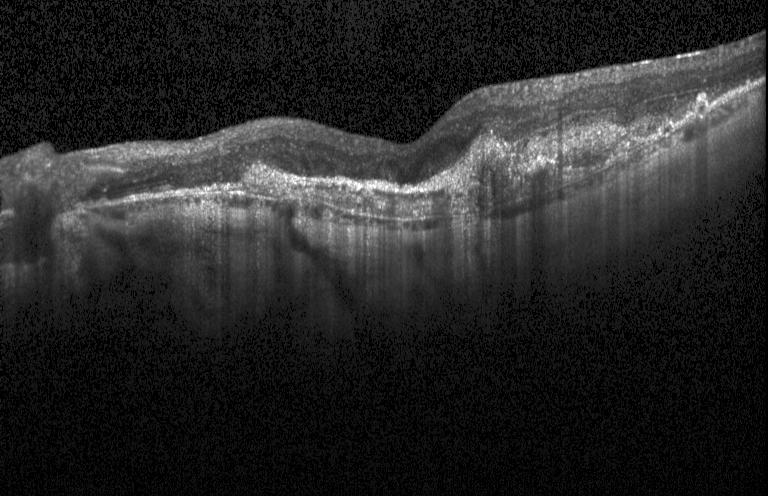 Retinal OCT cross-section · spectral-domain OCT.
Diagnosis: a choroidal neovascular membrane.